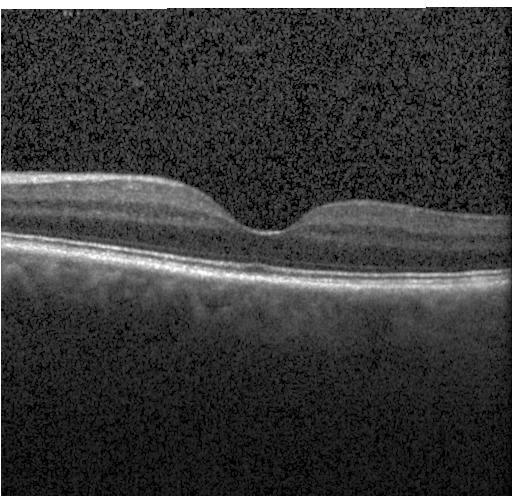

Optical coherence tomography B-scan. Macular scan. Acquired on a Heidelberg Spectralis. Spectral-domain OCT.
Impression: no choroidal neovascularization, diabetic macular edema, or drusen.